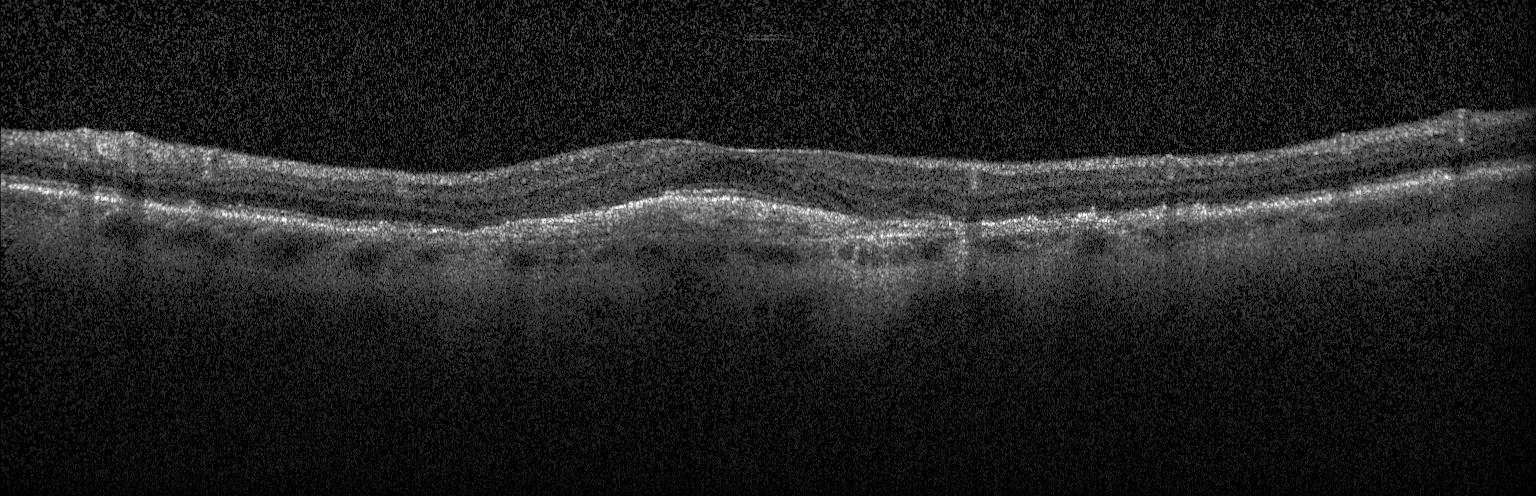
Acquired on a Heidelberg Spectralis · retinal OCT cross-section
Choroidal neovascularization.